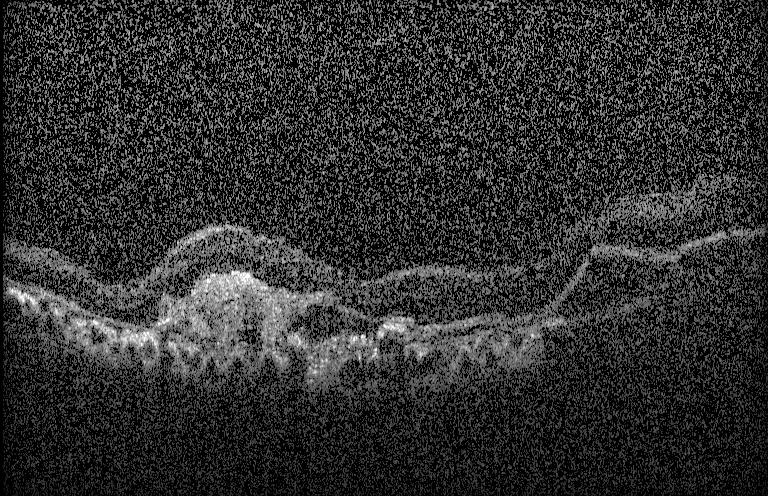 Optical coherence tomography scan
Impression: CNV.